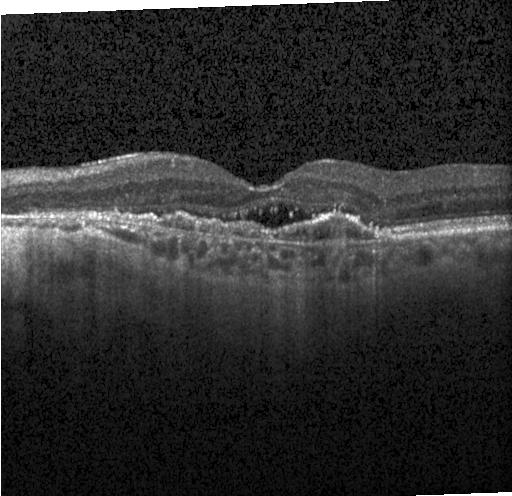 Optical coherence tomography scan; macular scan; Heidelberg Spectralis; spectral-domain OCT
A choroidal neovascular membrane.